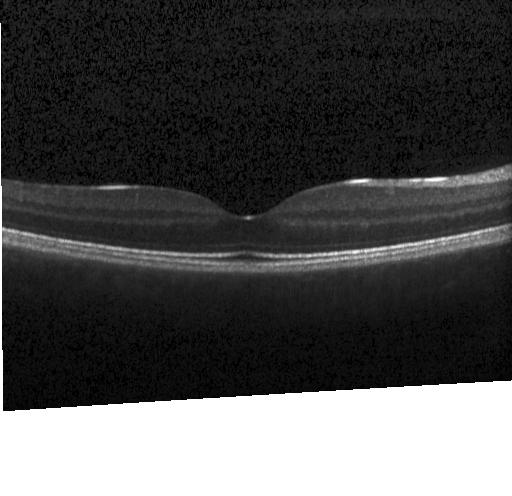

Finding: no evidence of choroidal neovascularization, diabetic macular edema, or drusen.